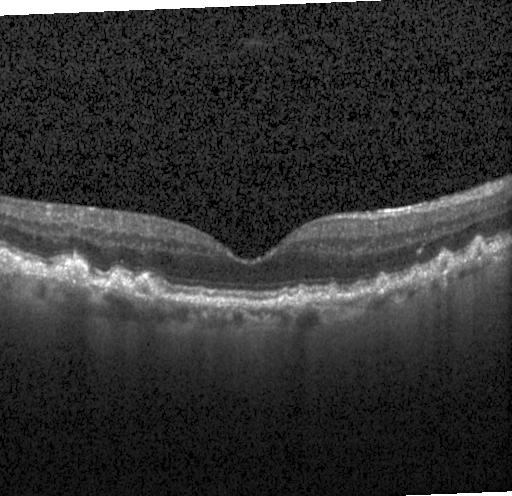 Macular scan, optical coherence tomography scan — Impression: drusen.